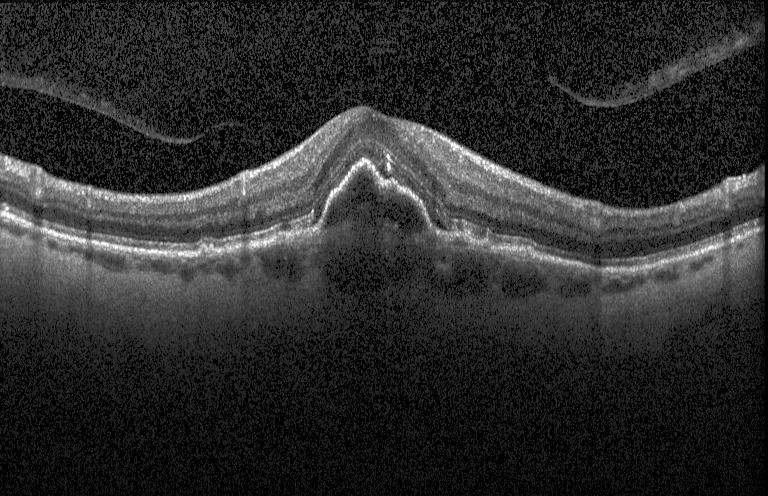 Dx: a choroidal neovascular membrane.